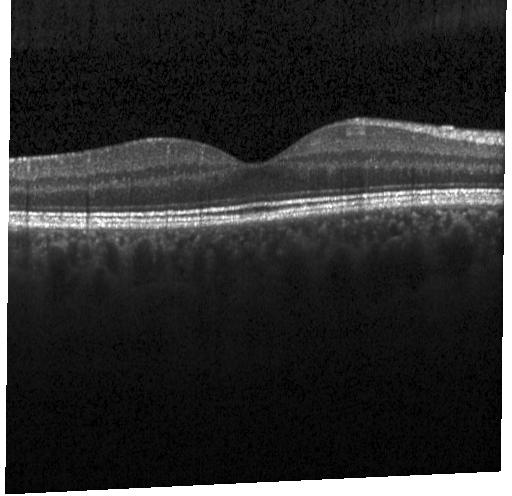

Retinal OCT B-scan. Spectral-domain OCT. Macular scan. Acquired on a Heidelberg Spectralis. Assessment: no evidence of choroidal neovascularization, diabetic macular edema, or drusen.